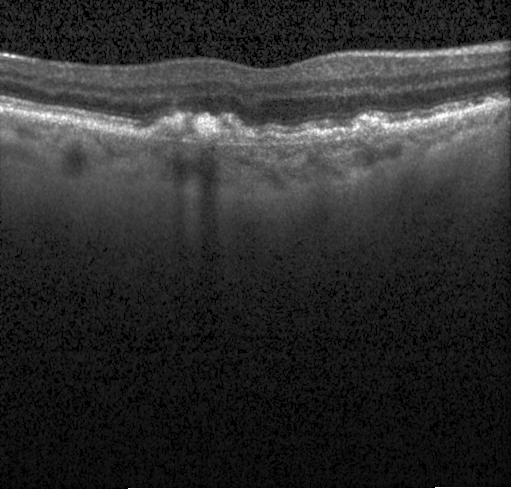
Horizontal scan through the fovea. Acquired on a Heidelberg Spectralis. Optical coherence tomography scan
Finding: choroidal neovascularization (CNV).